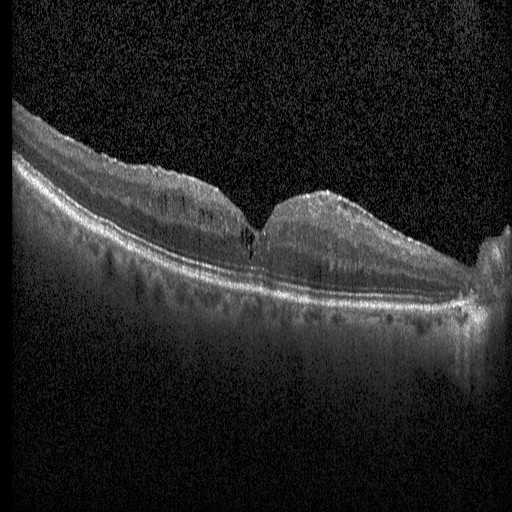 Acquired on a Heidelberg Spectralis · optical coherence tomography scan.
Finding: diabetic macular edema.